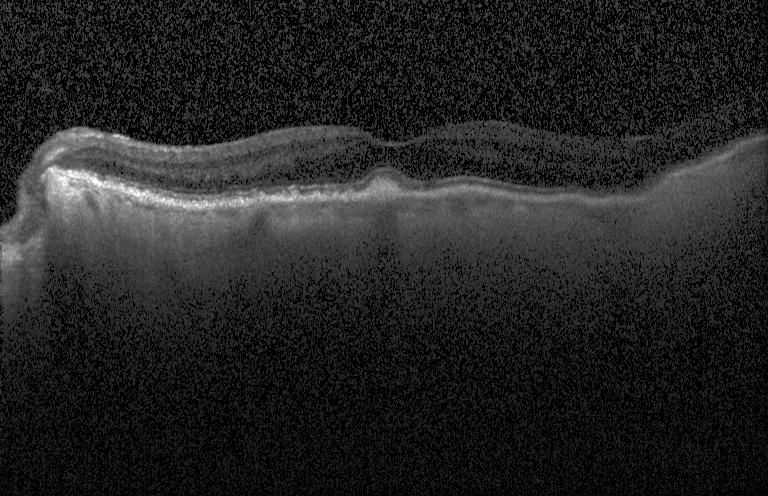
Optical coherence tomography scan
Macular OCT: multiple drusen.